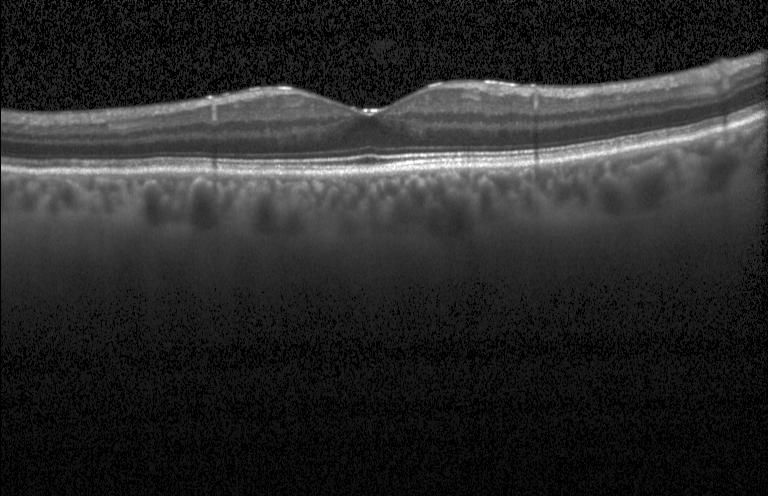
Retinal OCT cross-section.
Diagnosis: no choroidal neovascularization, diabetic macular edema, or drusen.